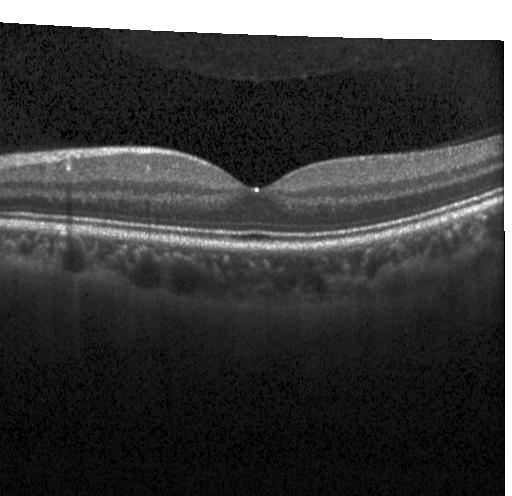 Retinal OCT B-scan
Diagnosis: no choroidal neovascularization, no diabetic macular edema, and no drusen.